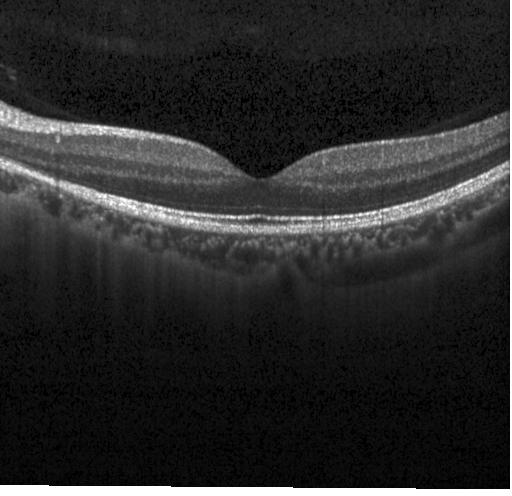

Macular OCT demonstrating no CNV, no DME, and no drusen.